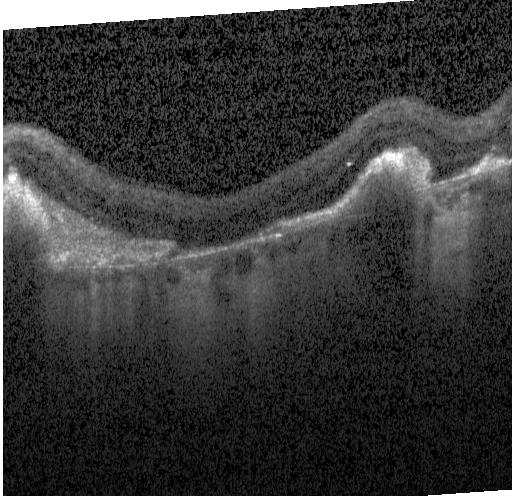
Optical coherence tomography scan. Finding: a choroidal neovascular membrane.